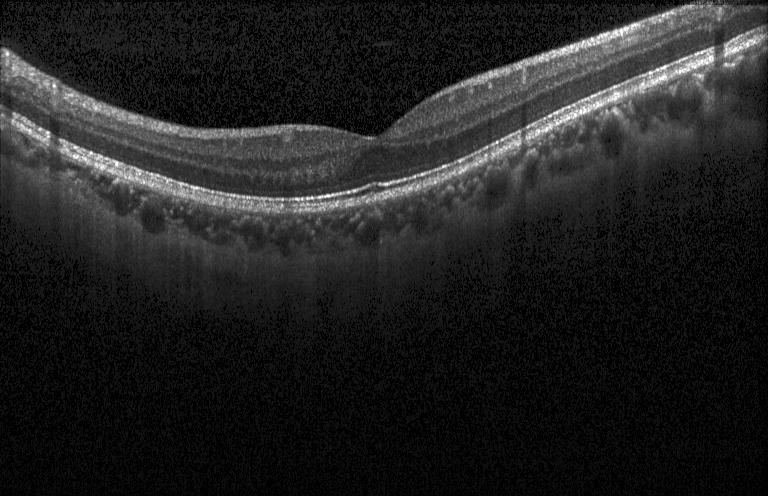
Macular OCT: no evidence of CNV, DME, or drusen.